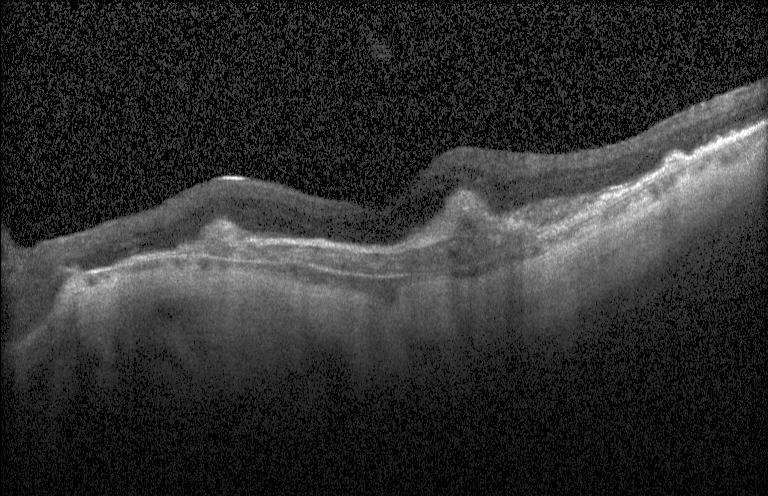
Instrument: Heidelberg Spectralis; OCT B-scan; spectral-domain OCT. Finding: a choroidal neovascular membrane.